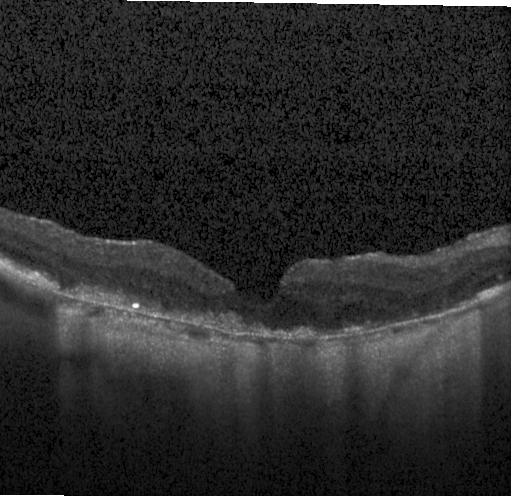
Retinal OCT cross-section. Heidelberg Spectralis OCT system. Finding: a choroidal neovascular membrane.